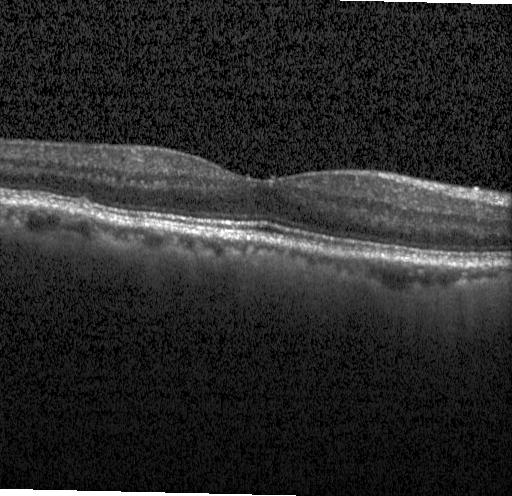 Acquired on a Heidelberg Spectralis · spectral-domain OCT · retinal OCT B-scan · horizontal scan through the fovea
Impression: neither choroidal neovascularization, diabetic macular edema, nor drusen.